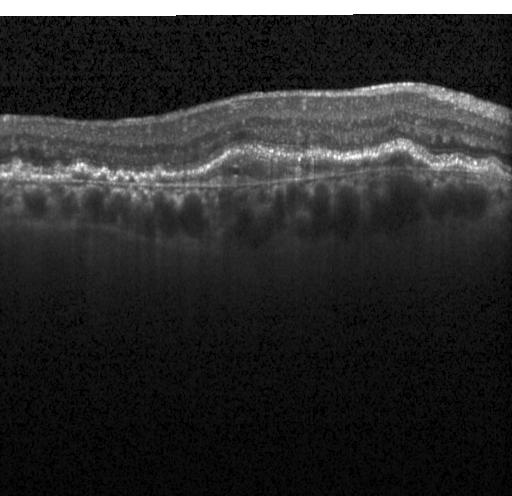

Spectral-domain OCT · optical coherence tomography scan · acquired on a Heidelberg Spectralis — The scan shows choroidal neovascularization.